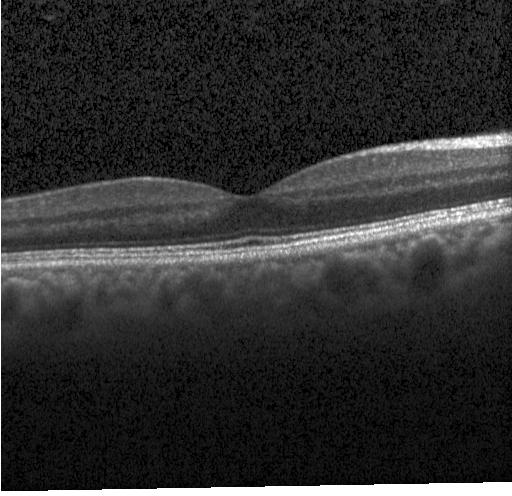
Finding: no evidence of CNV, DME, or drusen.